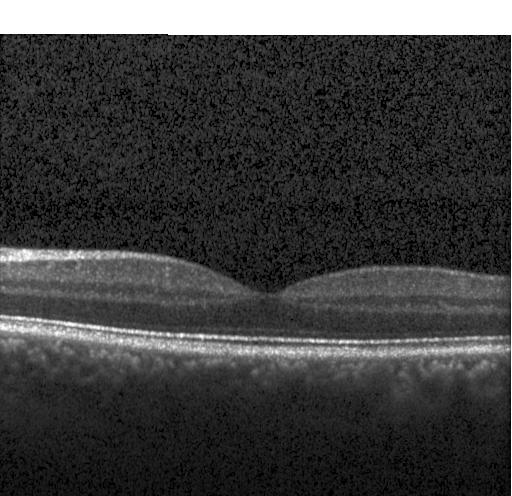 OCT line scan. Instrument: Heidelberg Spectralis. SD-OCT — Finding: no CNV, DME, or drusen.